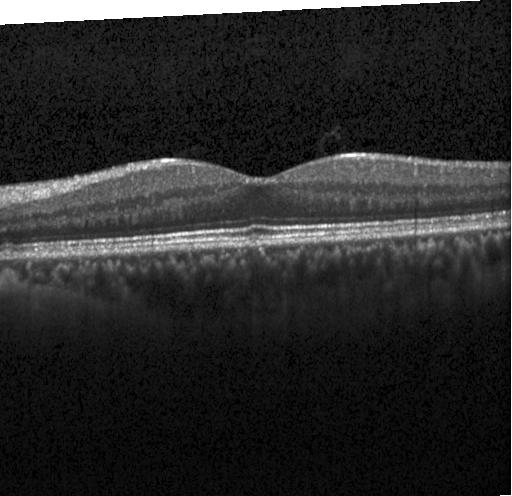

This B-scan demonstrates no choroidal neovascularization, diabetic macular edema, or drusen.